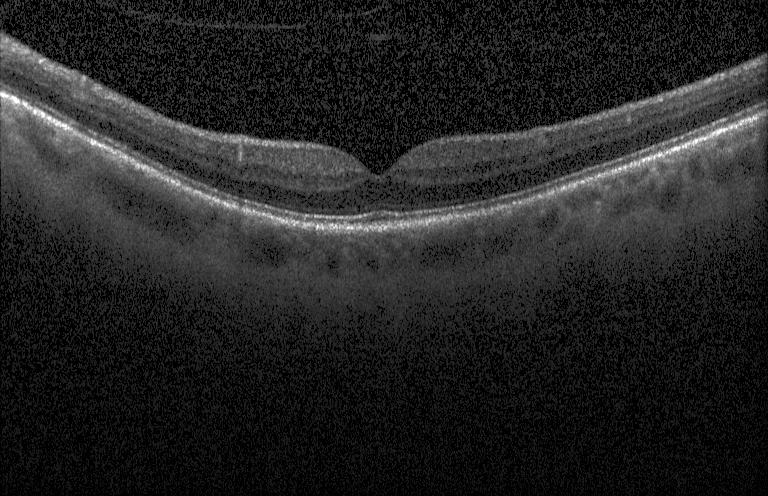

Optical coherence tomography B-scan. Impression: no choroidal neovascularization, no diabetic macular edema, and no drusen.